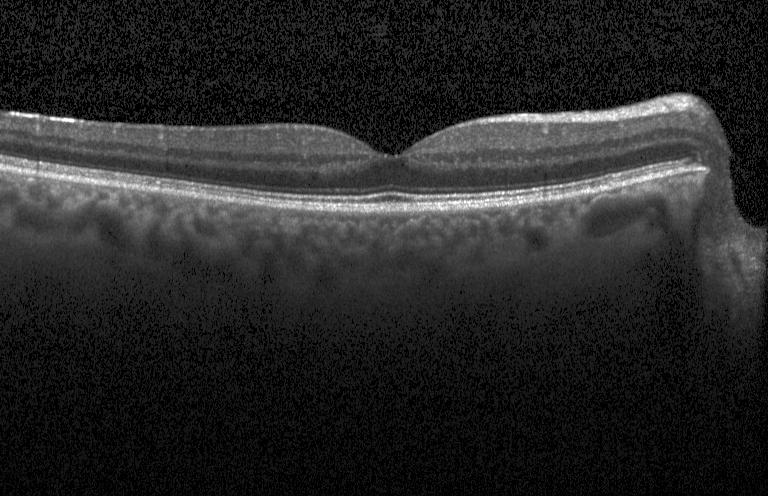
SD-OCT. OCT B-scan. Horizontal scan through the fovea. Acquired on a Heidelberg Spectralis. Impression: no evidence of choroidal neovascularization, diabetic macular edema, or drusen.